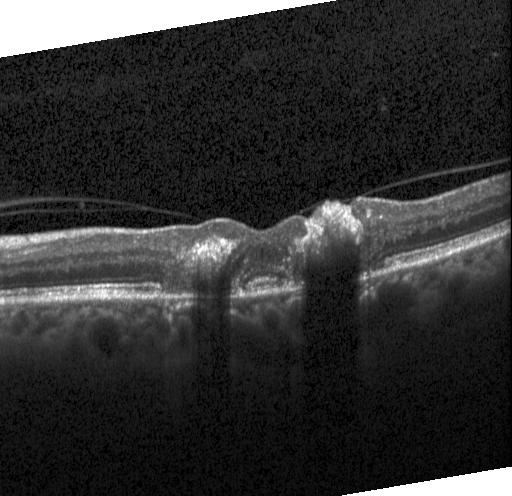
Retinal OCT B-scan
The scan shows choroidal neovascularization (CNV).